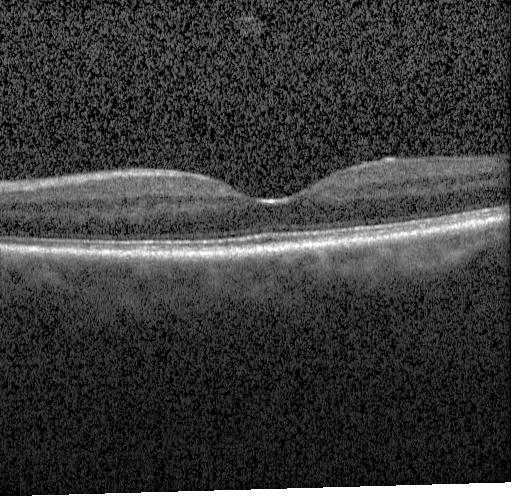 No CNV, no DME, and no drusen.